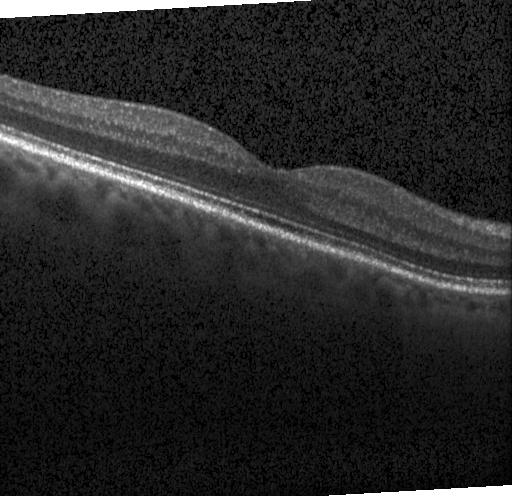

Dx: no CNV, DME, or drusen.